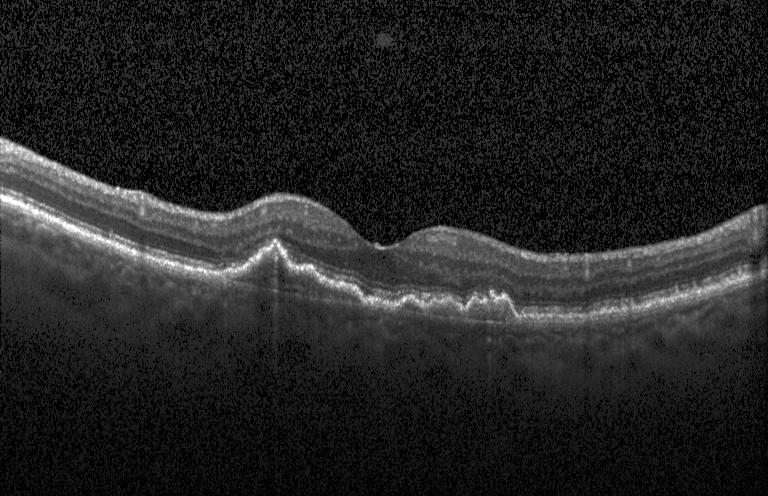 Spectral-domain OCT B-scan: CNV.